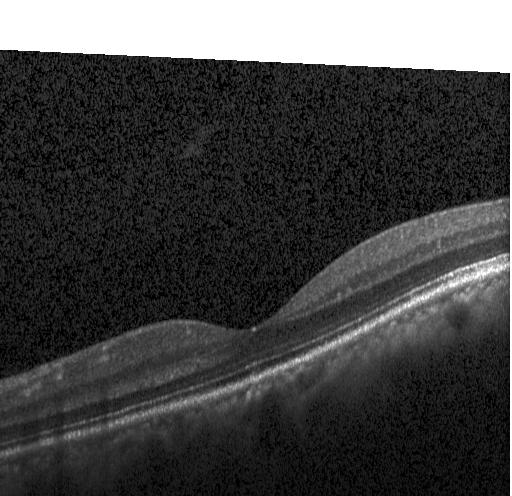 OCT B-scan showing no CNV, DME, or drusen.